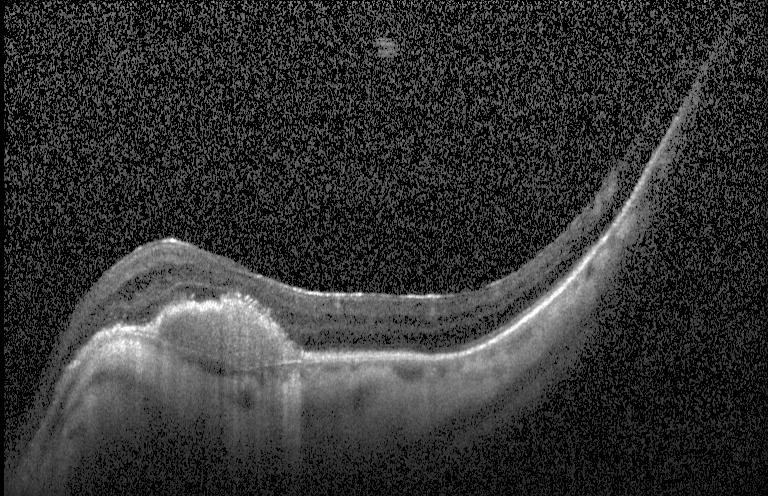

Finding: a choroidal neovascular membrane.